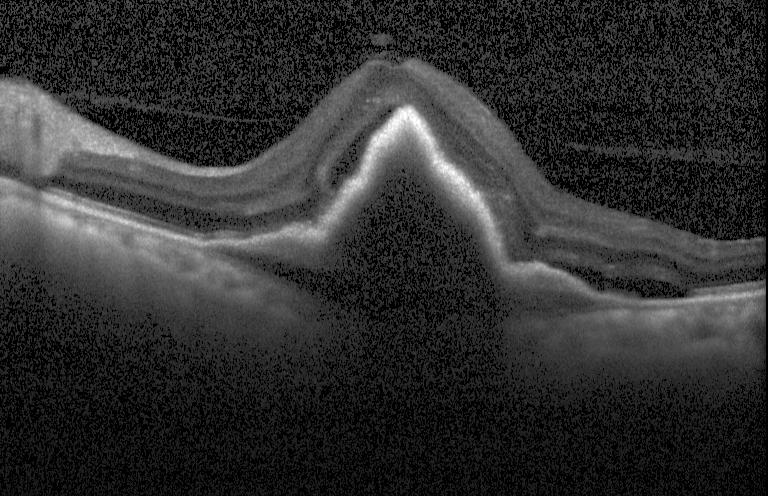

Impression: a choroidal neovascular membrane.